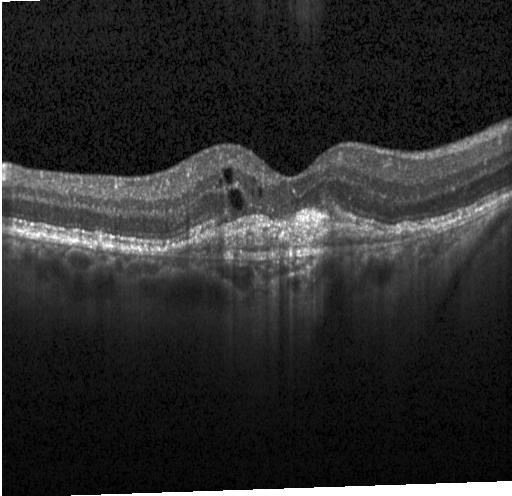

A choroidal neovascular membrane.